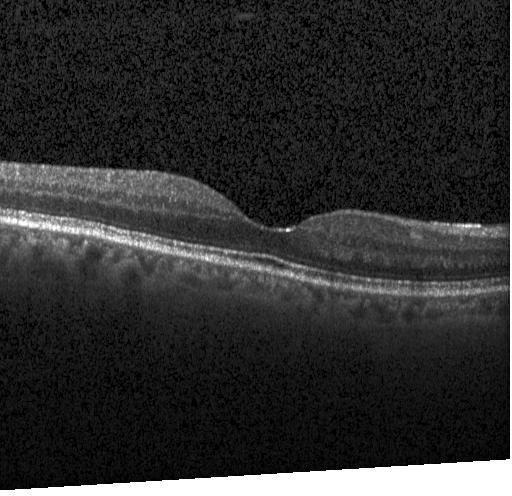 Finding: neither CNV, DME, nor drusen.